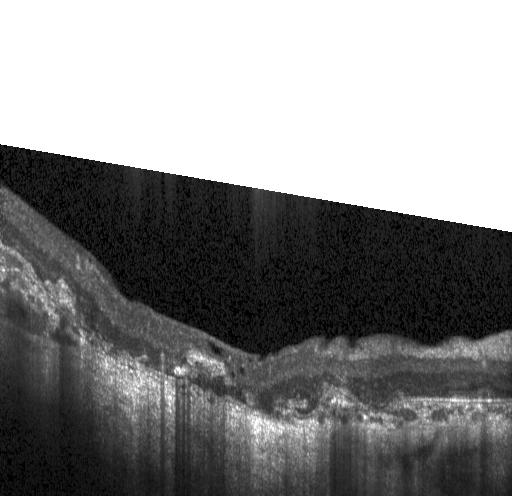
Macular OCT: a choroidal neovascular membrane.